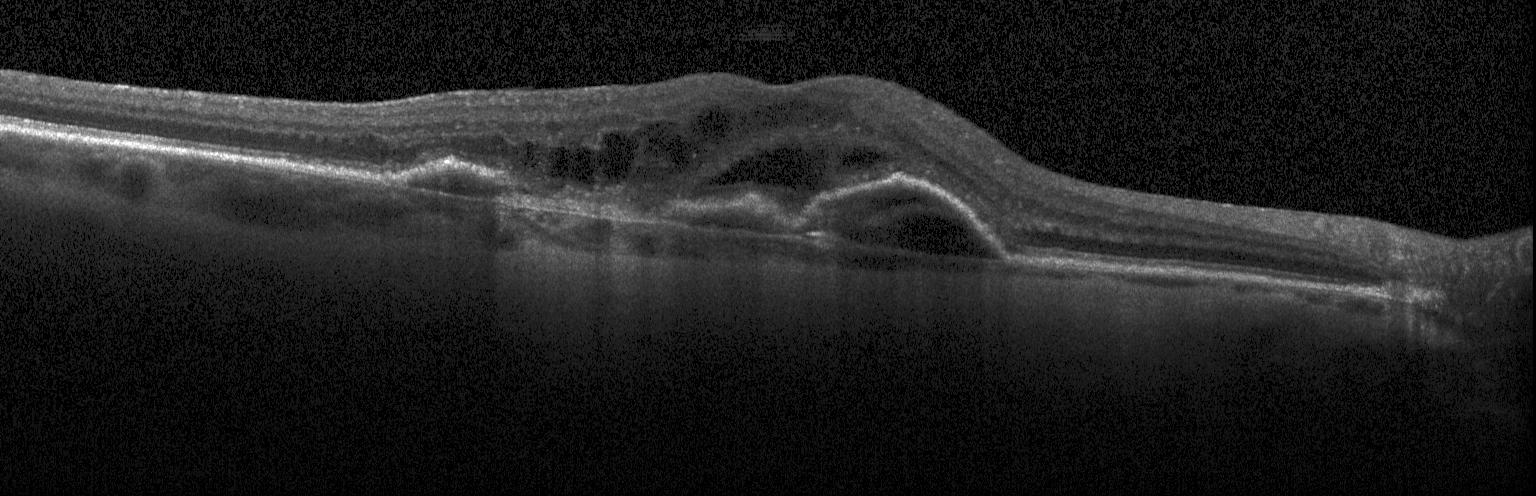

A choroidal neovascular membrane.